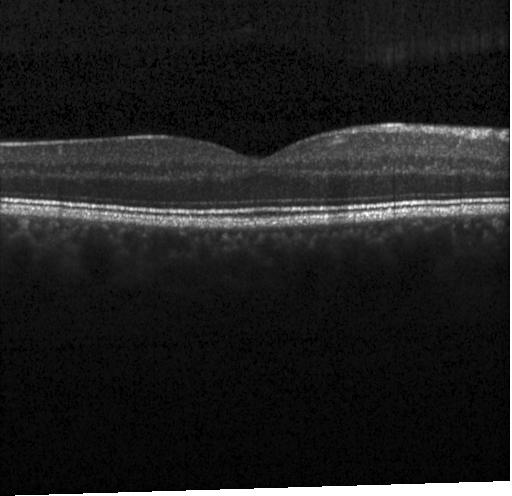 Retinal OCT B-scan · Heidelberg Spectralis OCT system — OCT finding: neither choroidal neovascularization, diabetic macular edema, nor drusen.